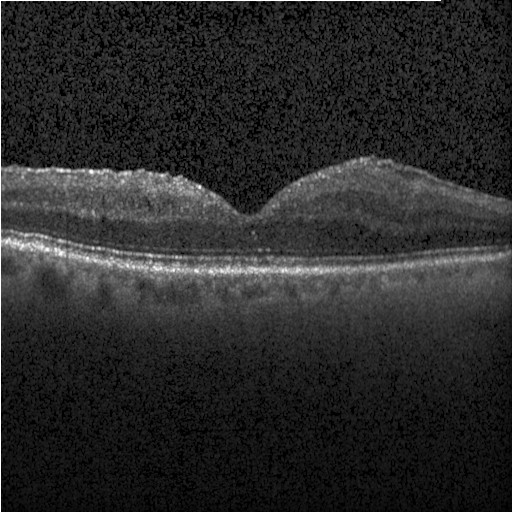

Impression: diabetic macular edema (DME).